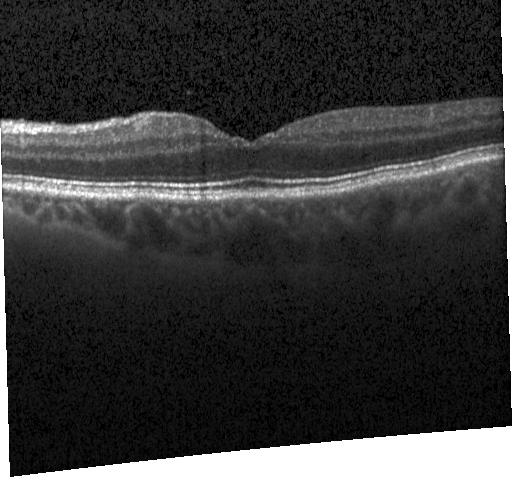
Impression: neither CNV, DME, nor drusen.